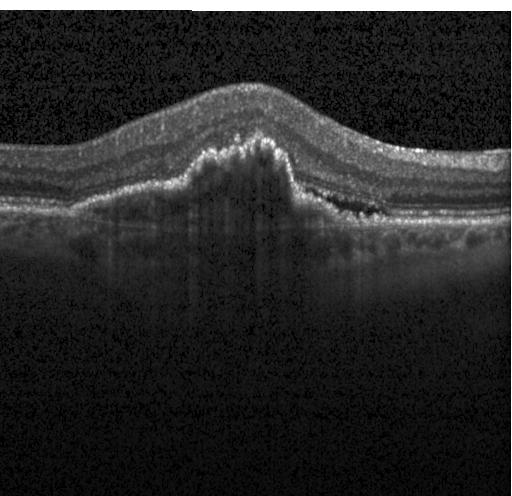 Acquired on a Heidelberg Spectralis. OCT line scan. Spectral-domain OCT. Horizontal scan through the fovea
Macular OCT: choroidal neovascularization.